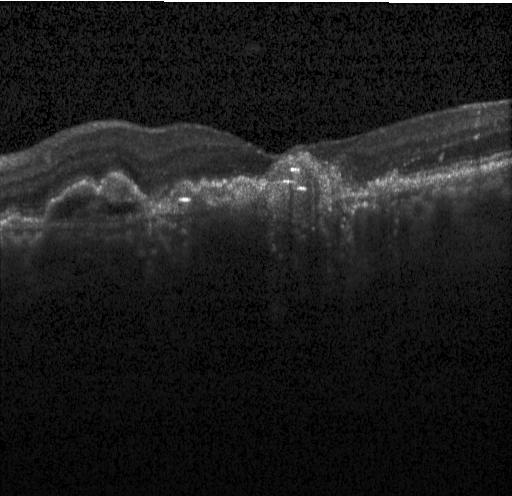
Through the macula, spectral-domain OCT, optical coherence tomography scan. Diagnosis: choroidal neovascularization (CNV).